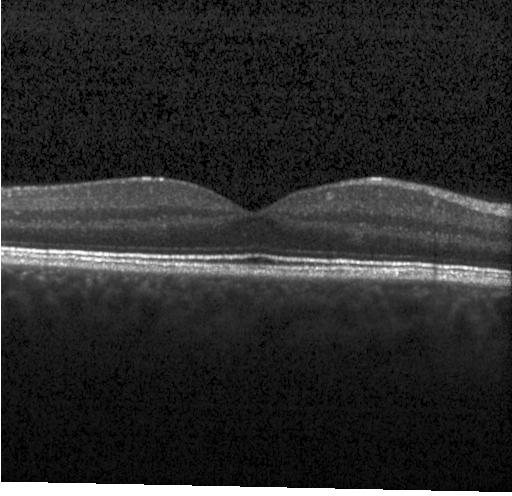
OCT line scan, centered on the fovea, SD-OCT, Heidelberg Spectralis.
OCT finding: neither CNV, DME, nor drusen.